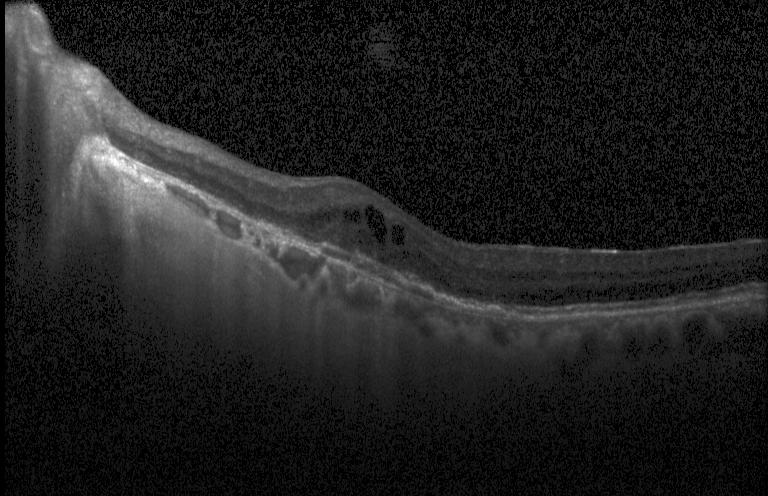

Retinal OCT cross-section. Impression: choroidal neovascularization.